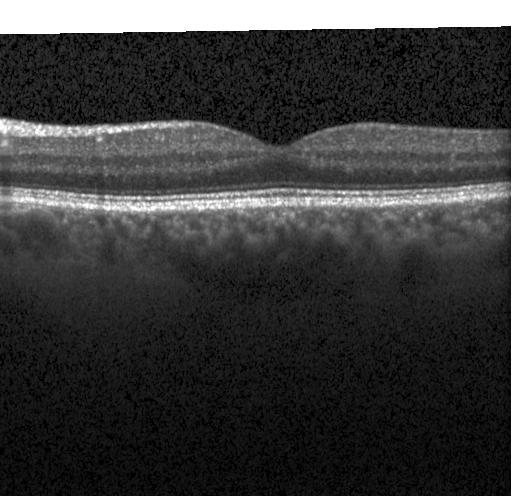
OCT scan showing no evidence of CNV, DME, or drusen.